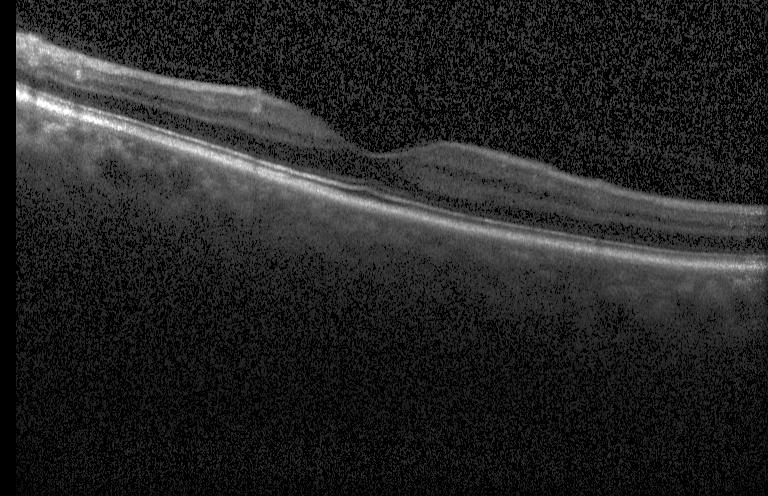

SD-OCT. Retinal OCT B-scan
OCT finding: no CNV, no DME, and no drusen.